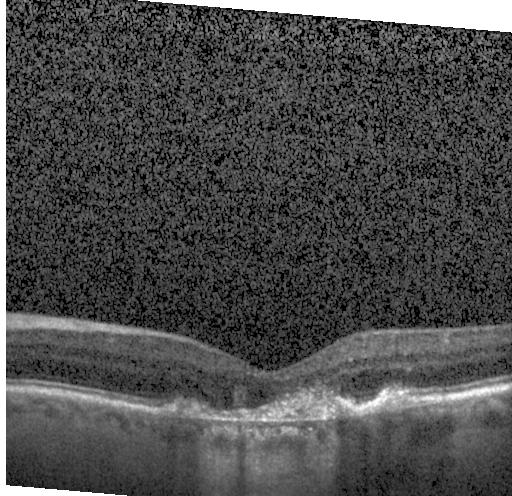 Retinal OCT cross-section. Impression: CNV.